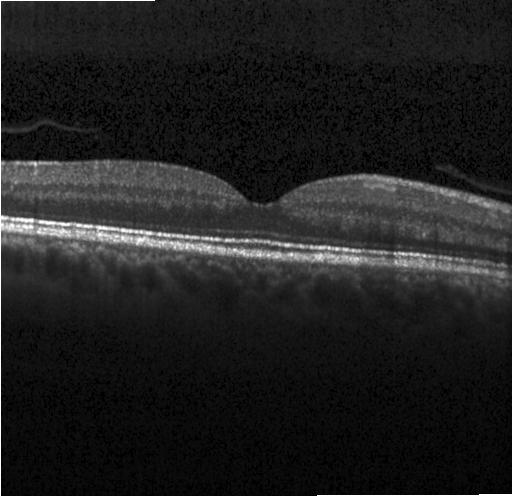 Horizontal scan through the fovea · Heidelberg Spectralis OCT system · OCT line scan · spectral-domain optical coherence tomography — Diagnosis: no choroidal neovascularization, no diabetic macular edema, and no drusen.